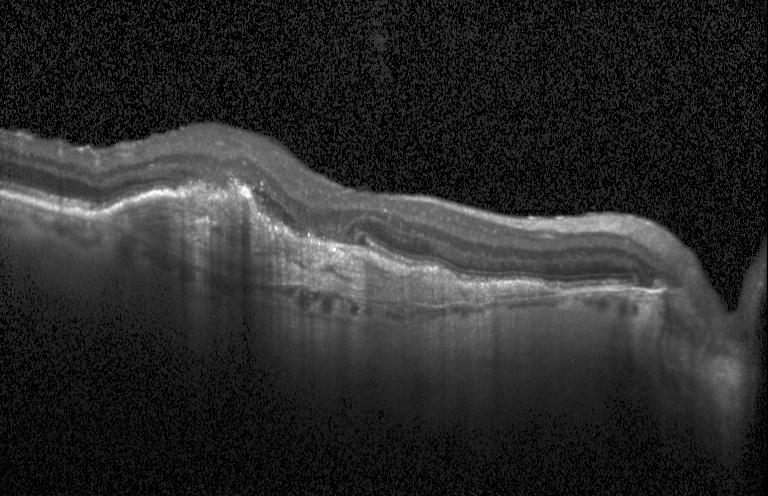
Instrument: Heidelberg Spectralis; optical coherence tomography scan. Diagnosis: choroidal neovascularization.